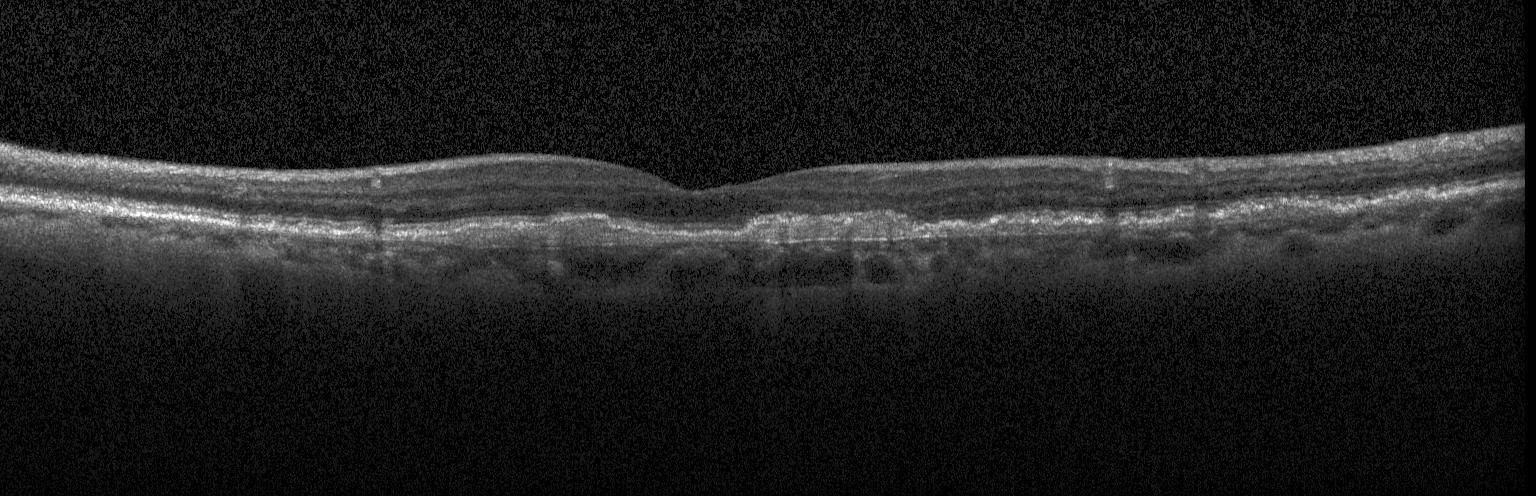
Finding: CNV.